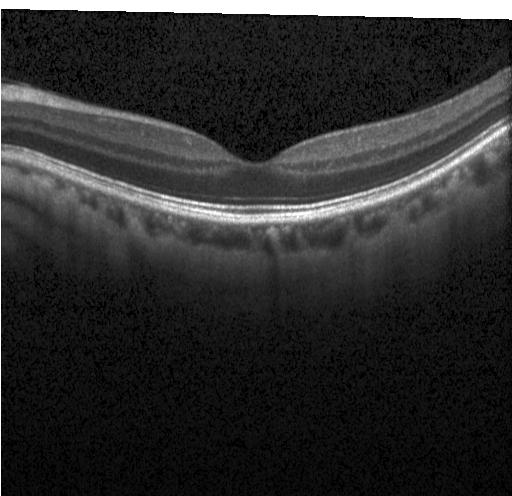
OCT line scan; fovea-centered — Assessment: neither CNV, DME, nor drusen.